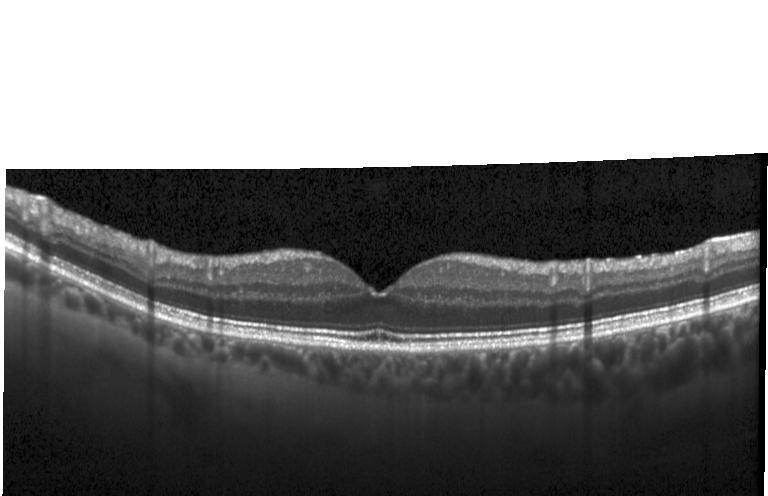

OCT finding: no choroidal neovascularization, no diabetic macular edema, and no drusen.